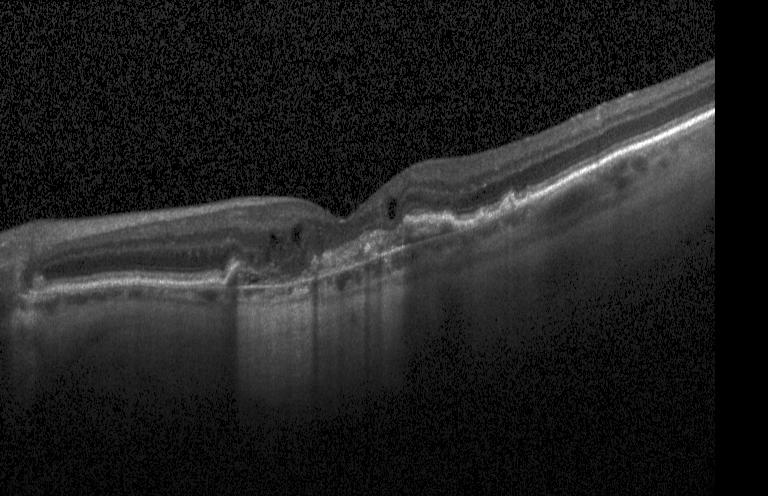
OCT scan showing a choroidal neovascular membrane.